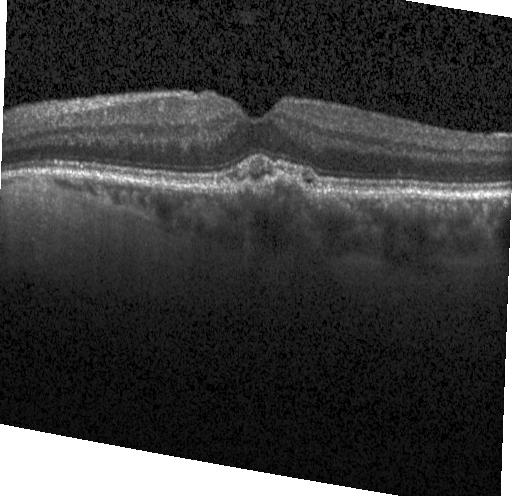
Dx: CNV.